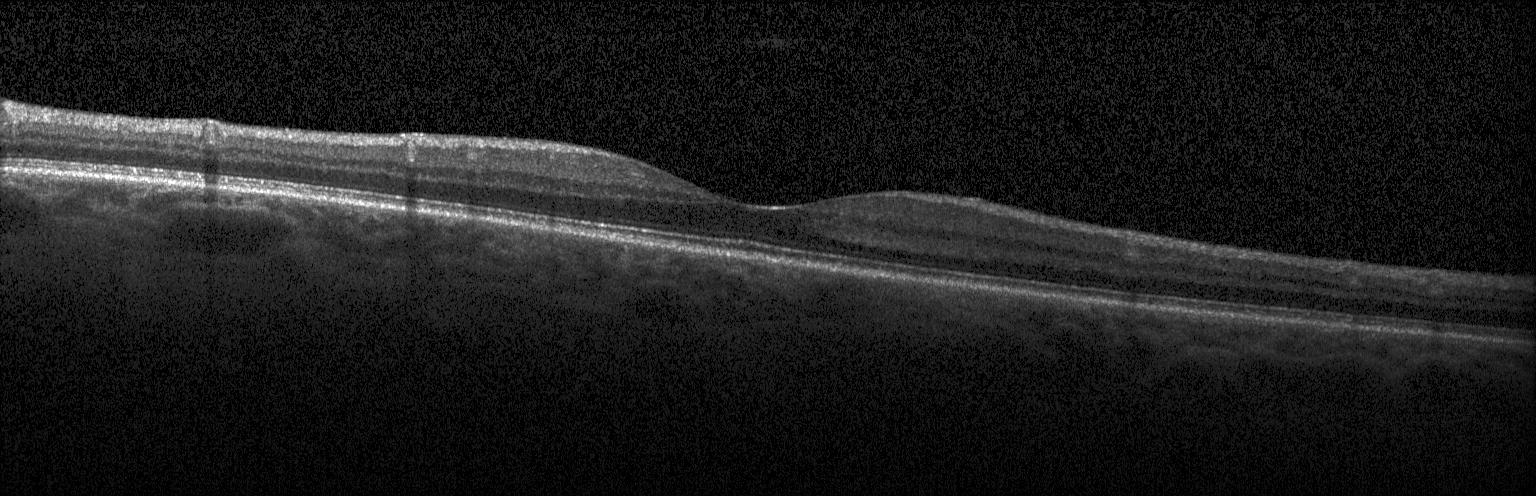

Optical coherence tomography scan, Heidelberg Spectralis OCT system, fovea-centered, SD-OCT.
OCT finding: no choroidal neovascularization, no diabetic macular edema, and no drusen.